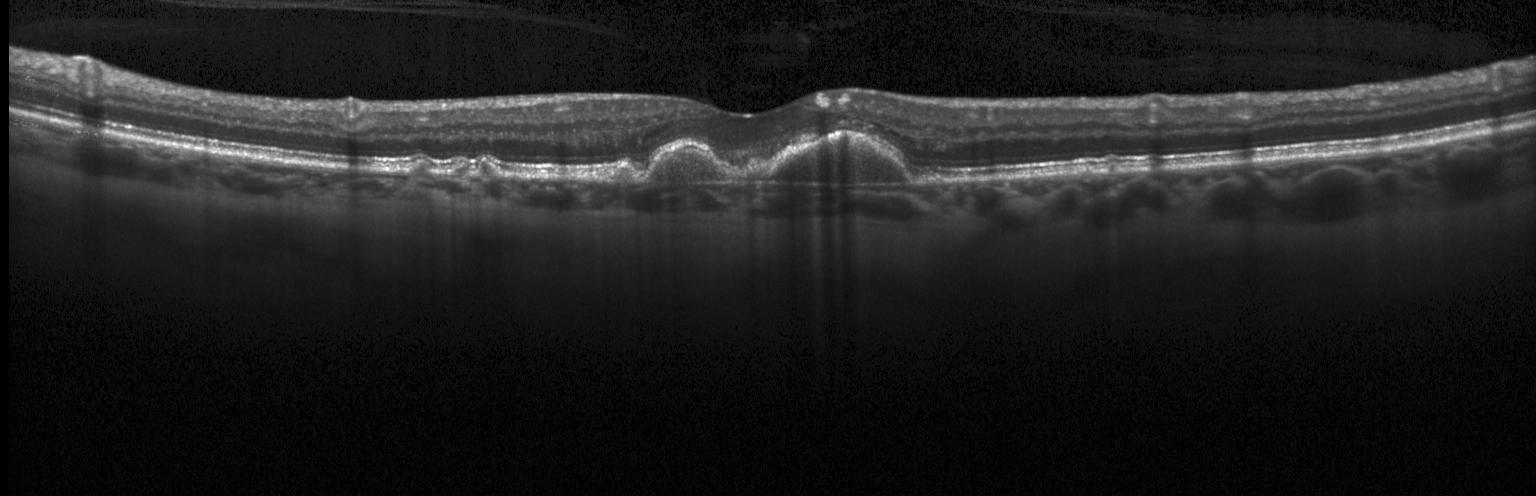
Optical coherence tomography B-scan; instrument: Heidelberg Spectralis.
Impression: a choroidal neovascular membrane.